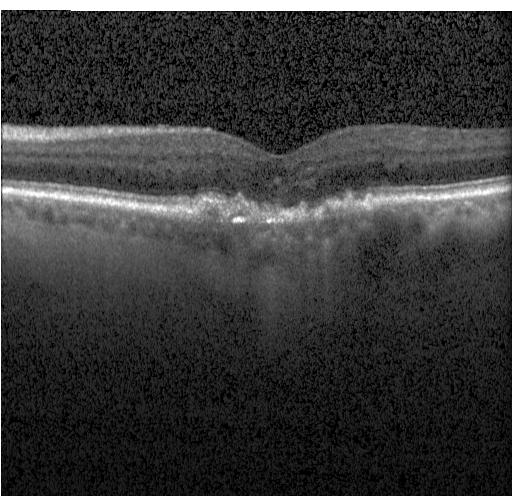

Choroidal neovascularization.